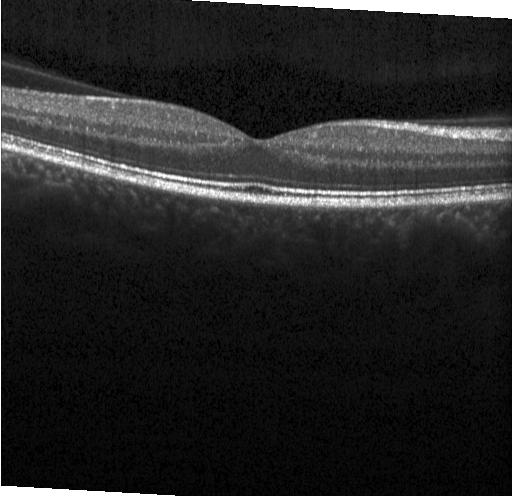

OCT line scan
The scan shows no evidence of choroidal neovascularization, diabetic macular edema, or drusen.